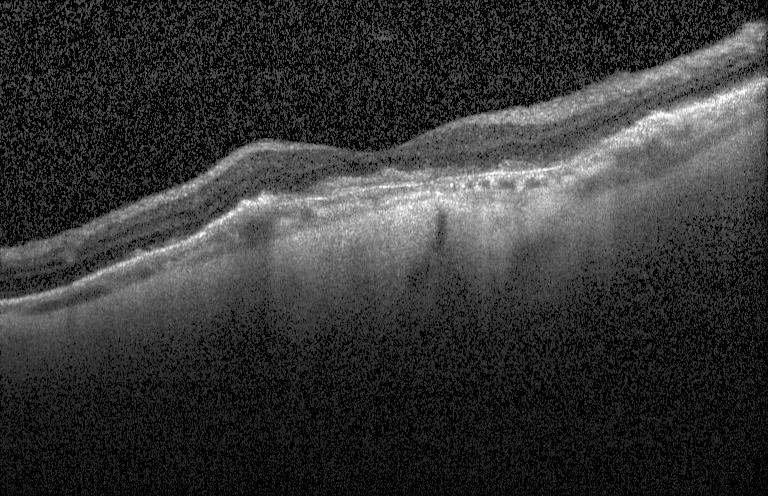
Retinal OCT B-scan. Acquired on a Heidelberg Spectralis
Diagnosis: choroidal neovascularization (CNV).